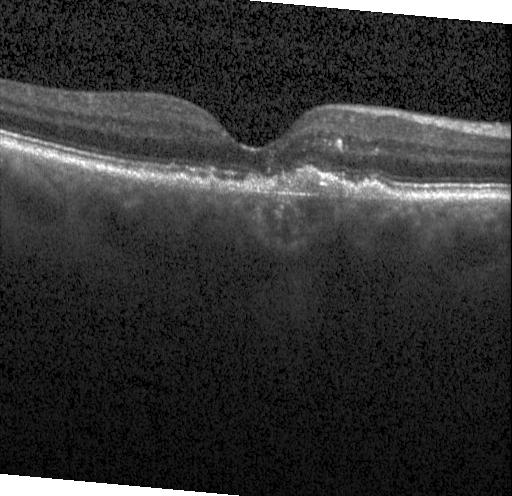
OCT B-scan — A choroidal neovascular membrane.